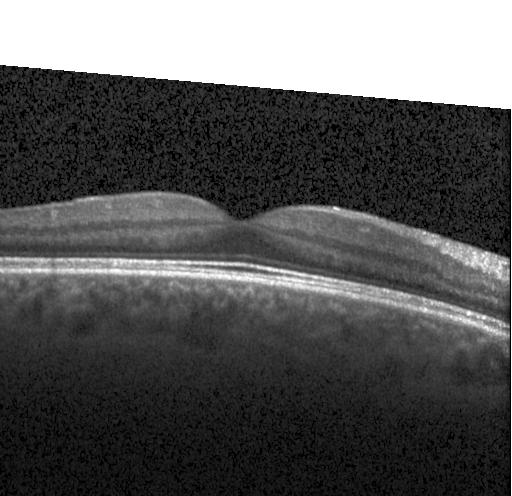
Acquired on a Heidelberg Spectralis; fovea-centered; retinal OCT B-scan.
Impression: neither CNV, DME, nor drusen.